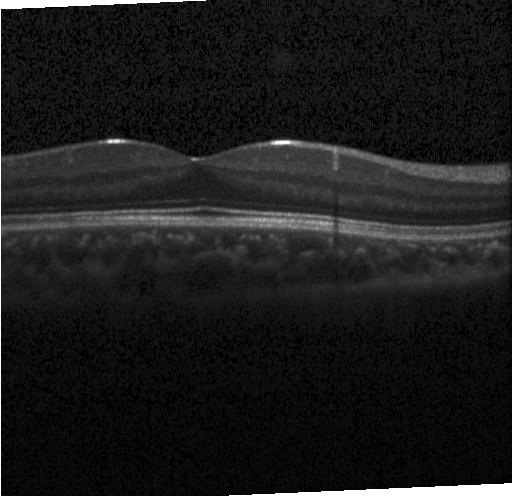

Acquired on a Heidelberg Spectralis; fovea-centered; retinal OCT cross-section. Dx: no choroidal neovascularization, no diabetic macular edema, and no drusen.